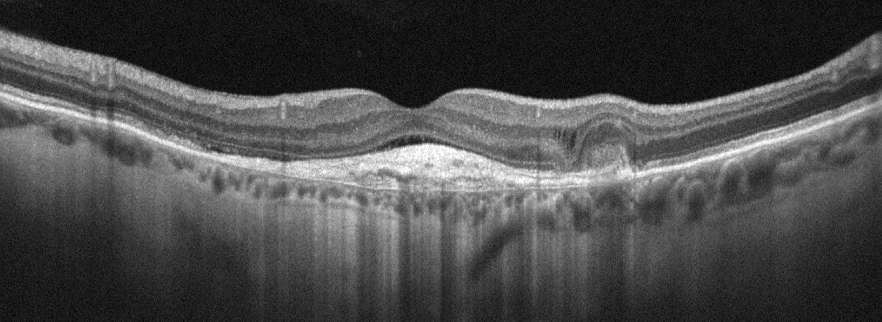 Oculus sinister; optical coherence tomography B-scan. This B-scan demonstrates age-related macular degeneration.